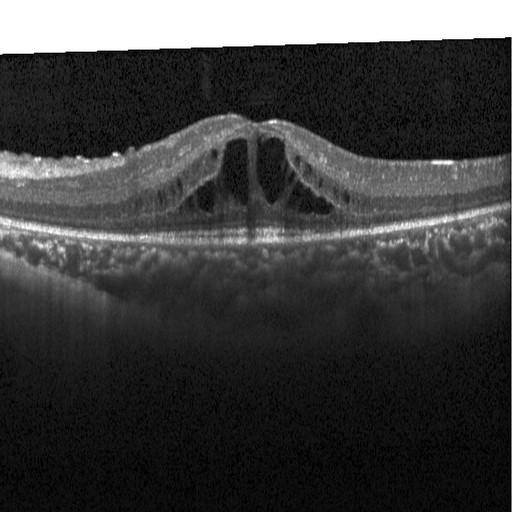
Assessment: diabetic macular edema (DME).